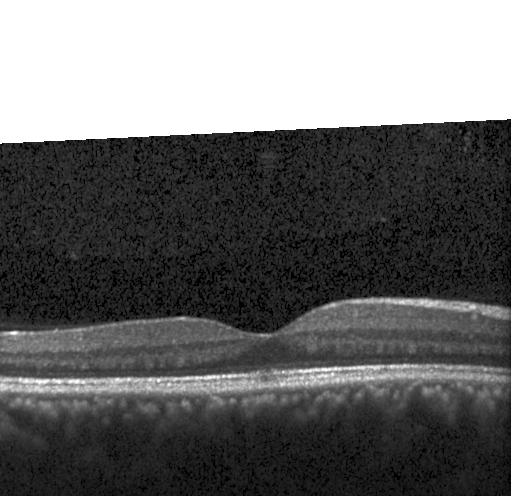
OCT line scan. Finding: neither choroidal neovascularization, diabetic macular edema, nor drusen.